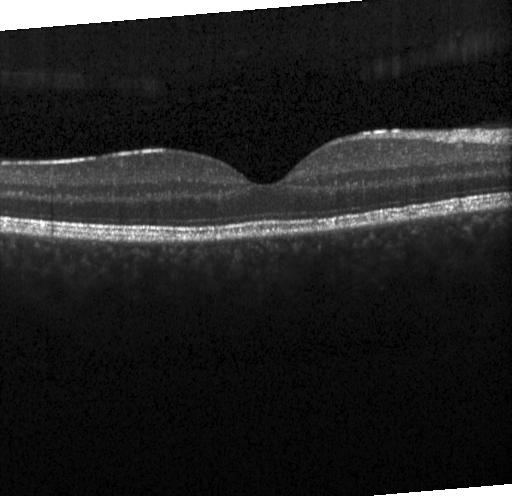
Retinal OCT cross-section · spectral-domain optical coherence tomography
Finding: no choroidal neovascularization, no diabetic macular edema, and no drusen.